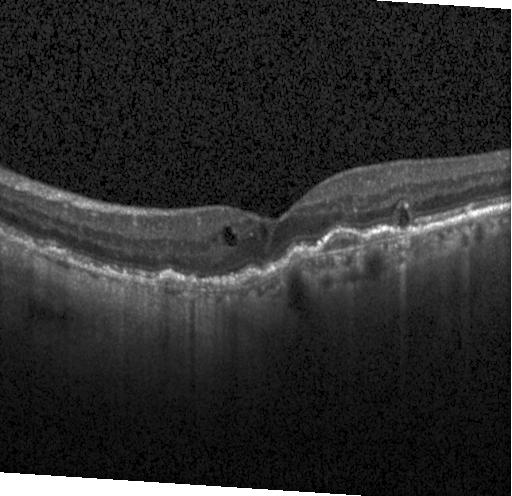
Impression: choroidal neovascularization.